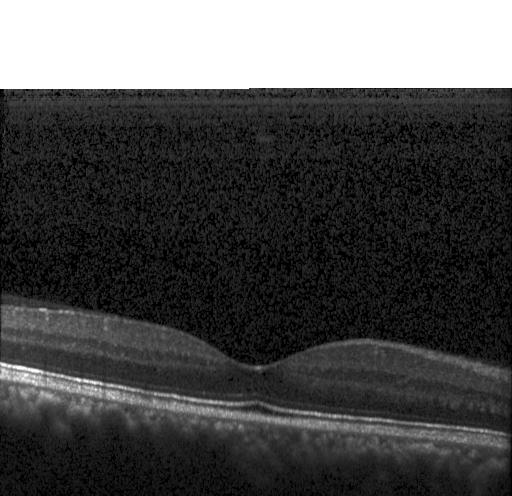 OCT B-scan, horizontal scan through the fovea.
No choroidal neovascularization, diabetic macular edema, or drusen.